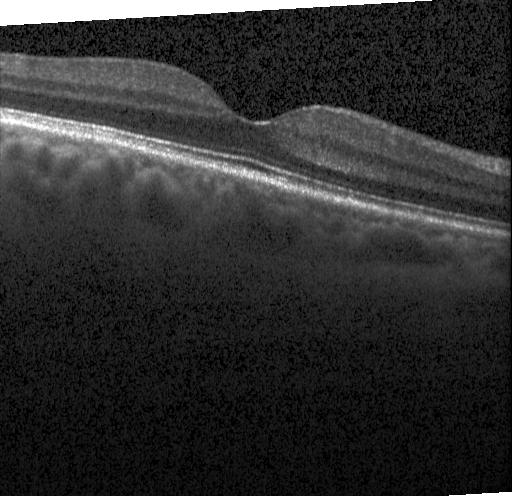 Impression: no choroidal neovascularization, no diabetic macular edema, and no drusen.